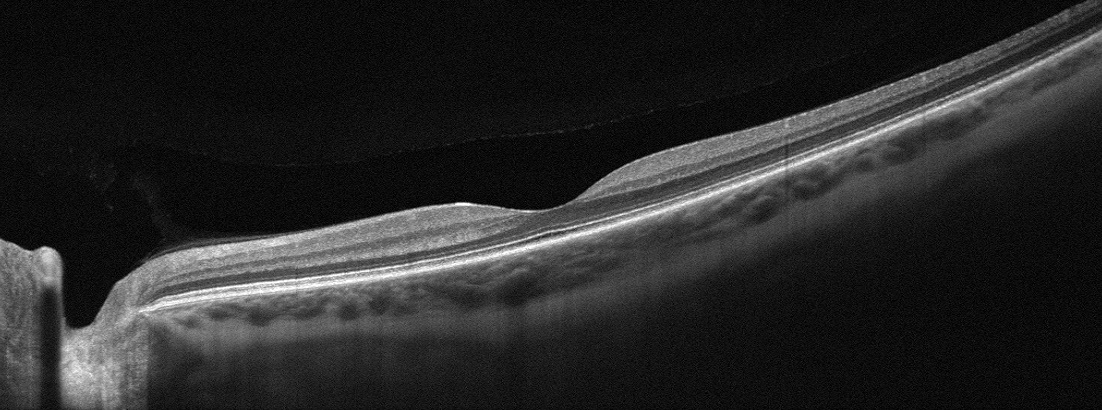
Instrument: Optovue Avanti RTVue XR · OCT B-scan
Assessment: no AMD, DME, ERM, RAO, RVO, or VID.